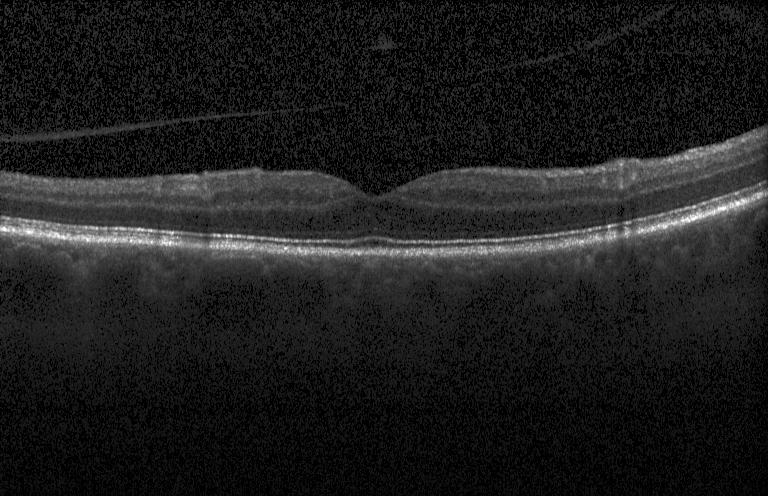 Retinal OCT cross-section · SD-OCT · acquired on a Heidelberg Spectralis · centered on the fovea. This B-scan demonstrates no choroidal neovascularization, no diabetic macular edema, and no drusen.